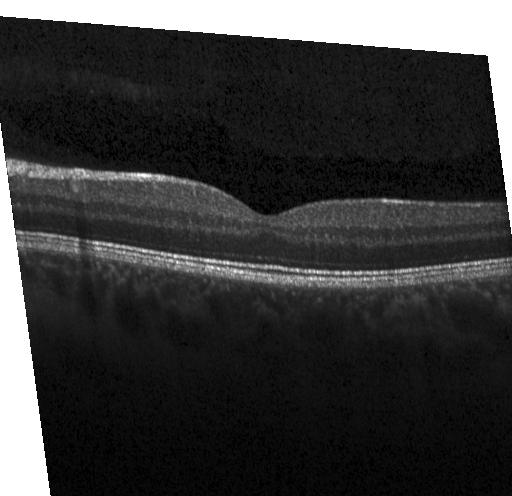
Fovea-centered; Heidelberg Spectralis; OCT B-scan — Finding: no choroidal neovascularization, diabetic macular edema, or drusen.